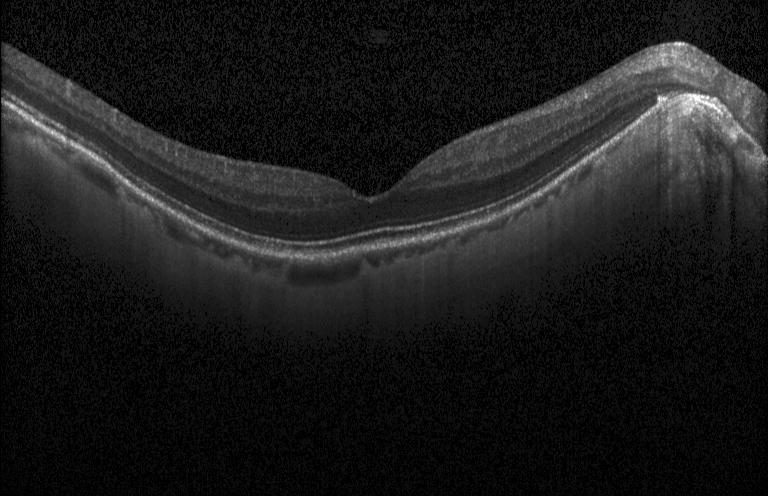
Dx: no choroidal neovascularization, diabetic macular edema, or drusen.